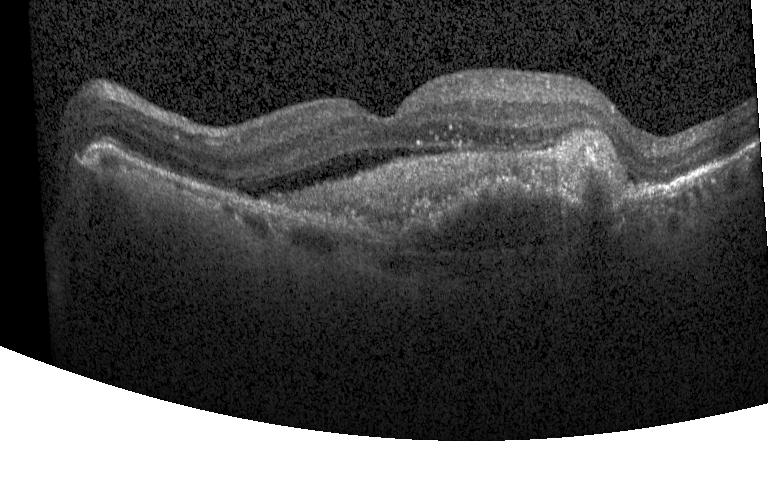 Macular OCT: choroidal neovascularization (CNV).